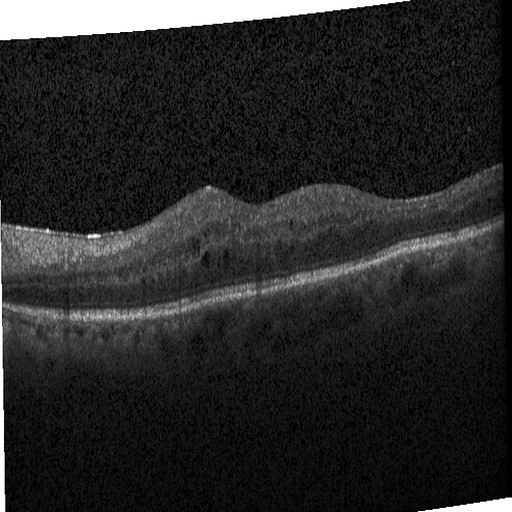

Impression: DME.